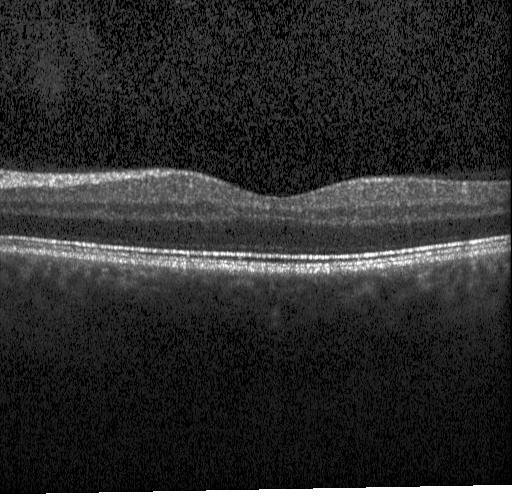 Macular scan, Heidelberg Spectralis OCT system, retinal OCT B-scan.
Impression: neither choroidal neovascularization, diabetic macular edema, nor drusen.